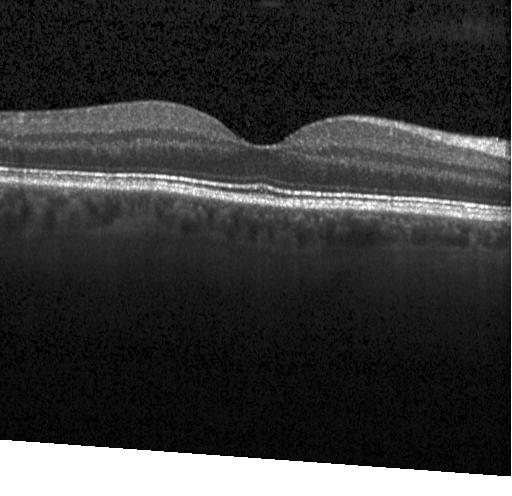
Optical coherence tomography B-scan
Finding: neither choroidal neovascularization, diabetic macular edema, nor drusen.